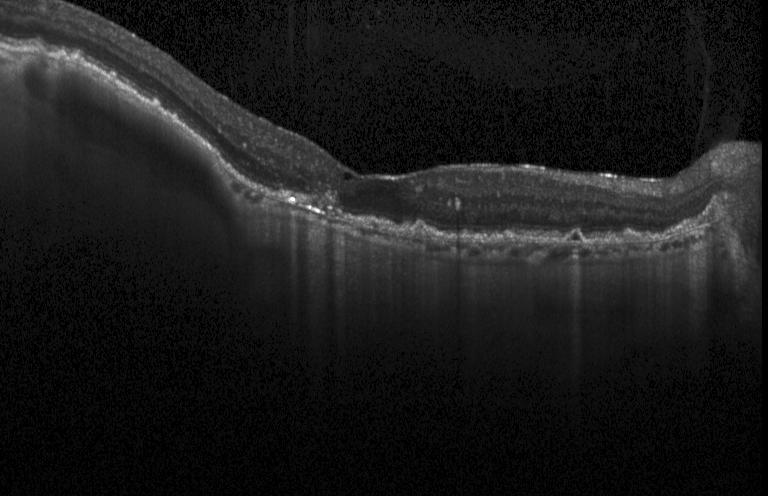

Spectral-domain optical coherence tomography. Optical coherence tomography B-scan. Acquired on a Heidelberg Spectralis — Diagnosis: choroidal neovascularization (CNV).